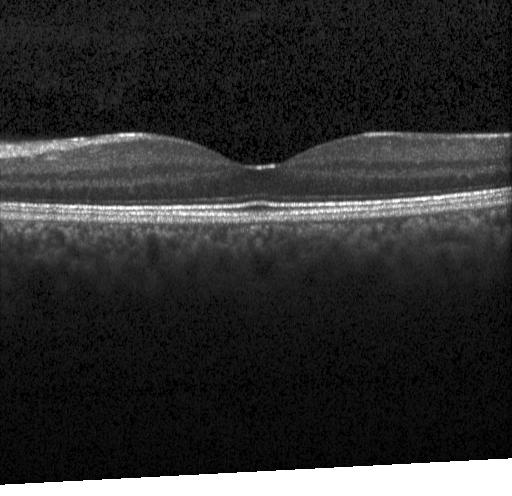 Spectral-domain OCT B-scan: no evidence of choroidal neovascularization, diabetic macular edema, or drusen.